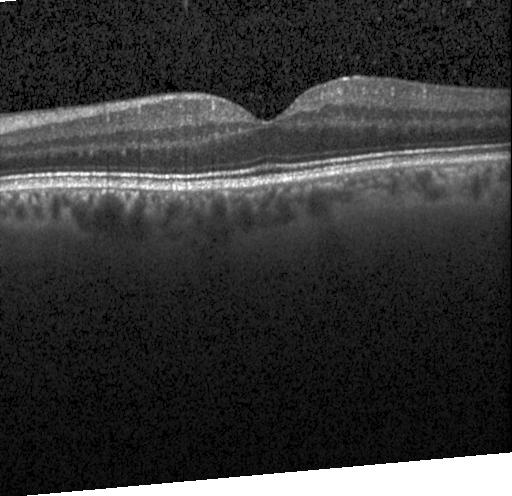

Diagnosis: no CNV, DME, or drusen.